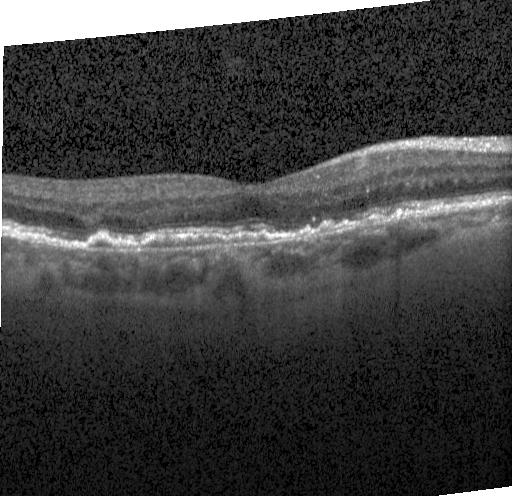 Retinal OCT B-scan · fovea-centered — OCT finding: CNV.